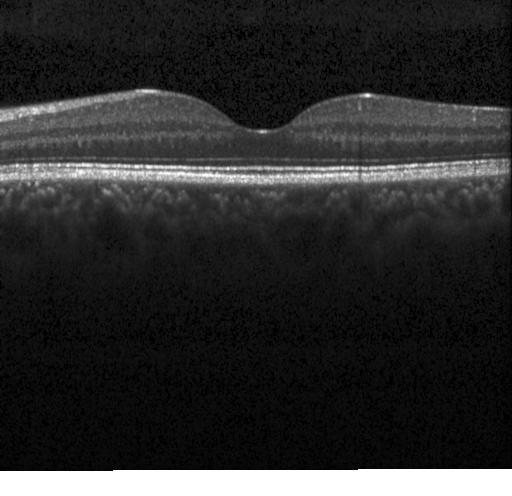

Optical coherence tomography scan · spectral-domain optical coherence tomography · fovea-centered
OCT finding: no choroidal neovascularization, no diabetic macular edema, and no drusen.